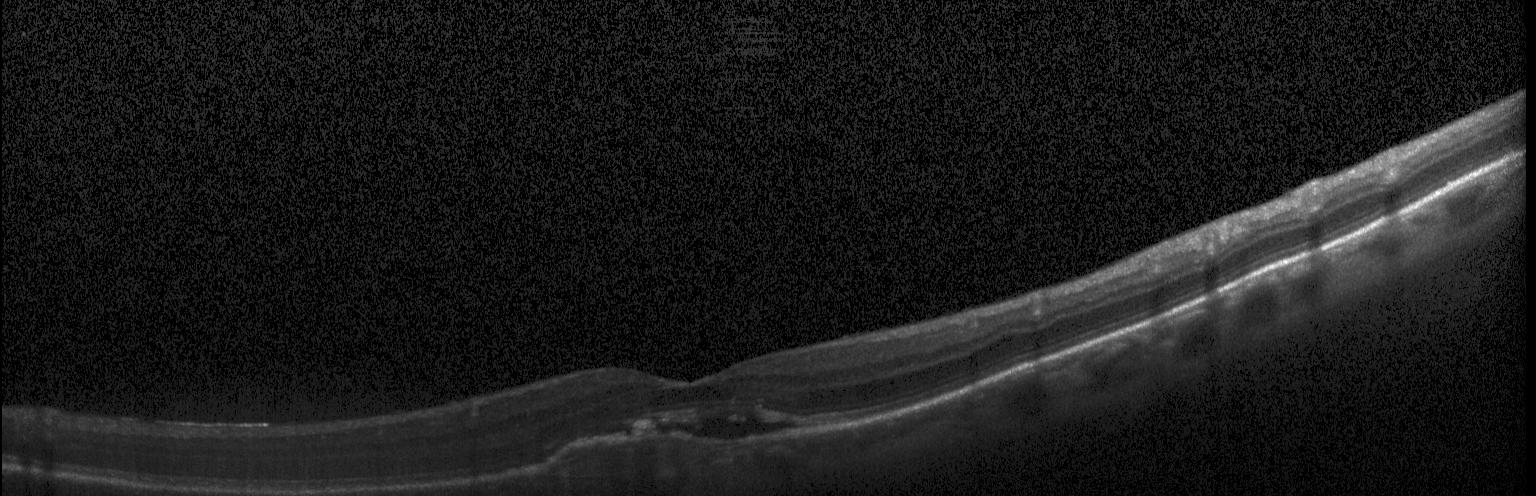 Through the macula; spectral-domain OCT; OCT line scan; instrument: Heidelberg Spectralis. This B-scan demonstrates a choroidal neovascular membrane.